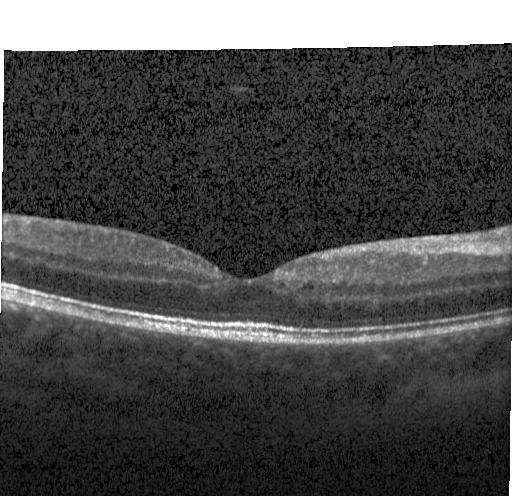 Spectral-domain OCT · optical coherence tomography B-scan · Heidelberg Spectralis · macular scan. Impression: diabetic macular edema (DME).